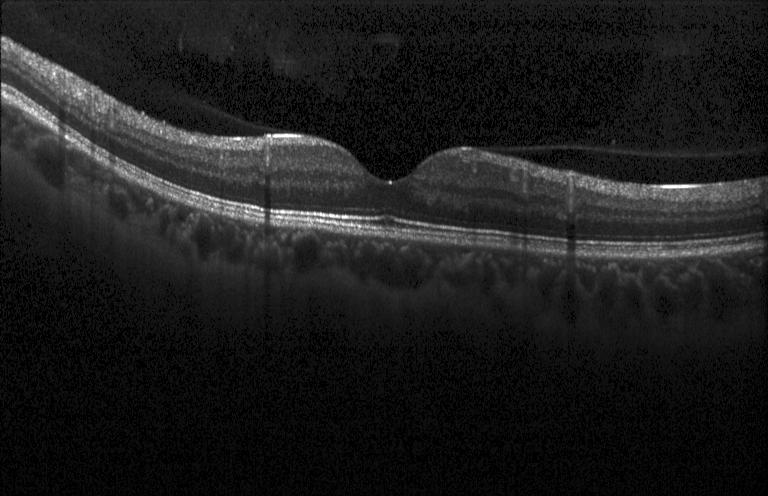

OCT line scan · SD-OCT
Finding: no CNV, DME, or drusen.